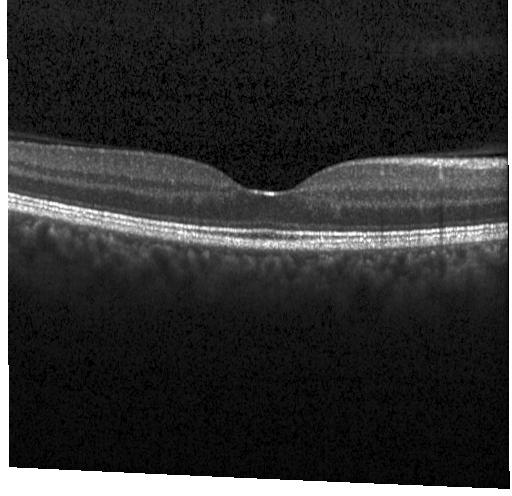
Optical coherence tomography B-scan · macular scan — Impression: neither choroidal neovascularization, diabetic macular edema, nor drusen.